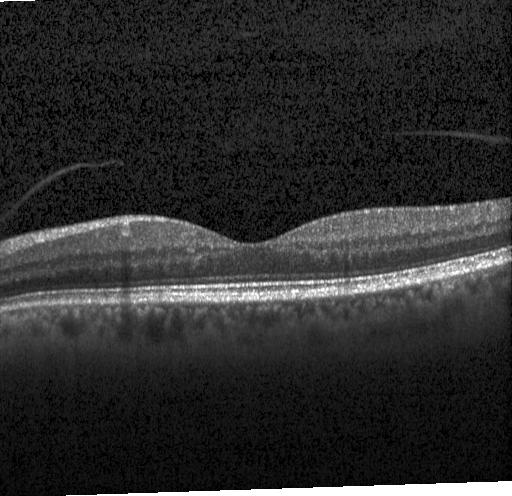
OCT B-scan. Spectral-domain OCT. Instrument: Heidelberg Spectralis. Through the macula.
This B-scan demonstrates no choroidal neovascularization, diabetic macular edema, or drusen.